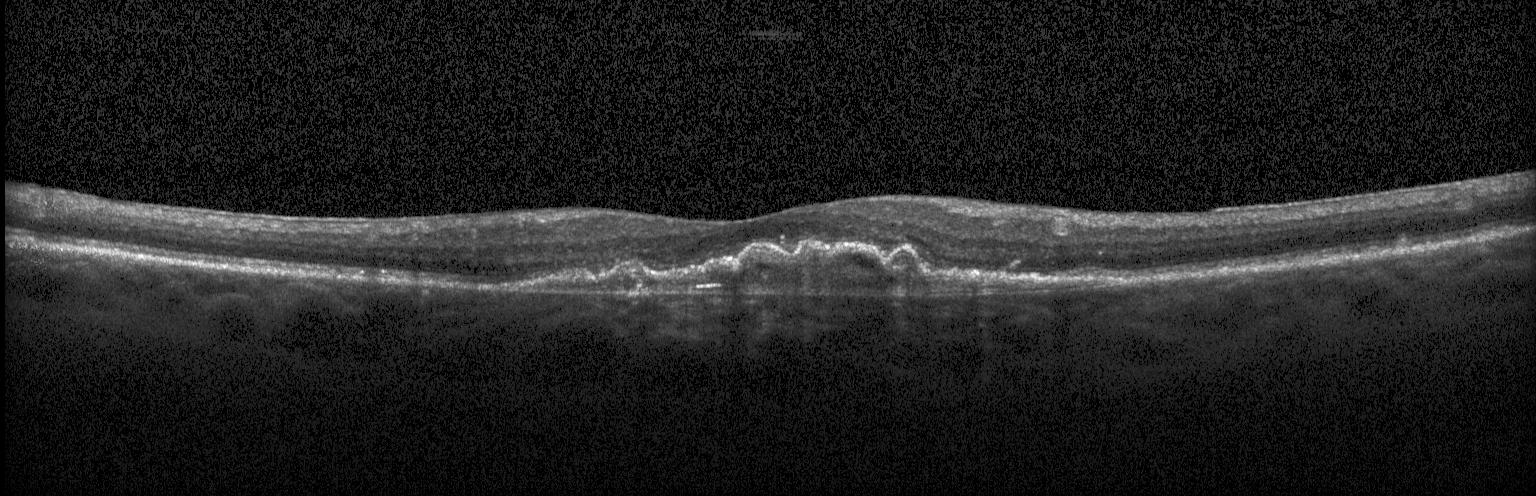

Optical coherence tomography B-scan. Spectral-domain optical coherence tomography.
Finding: a choroidal neovascular membrane.